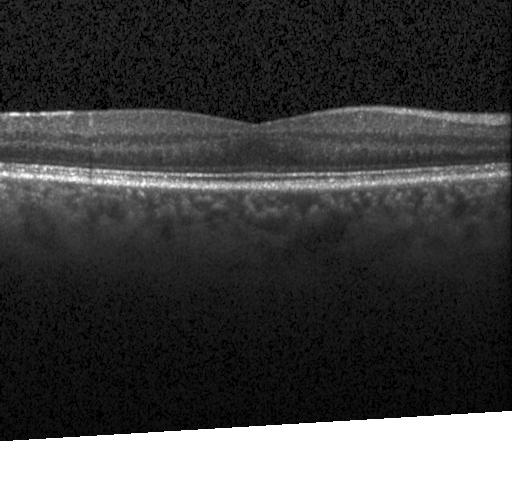
Macular OCT demonstrating neither choroidal neovascularization, diabetic macular edema, nor drusen.